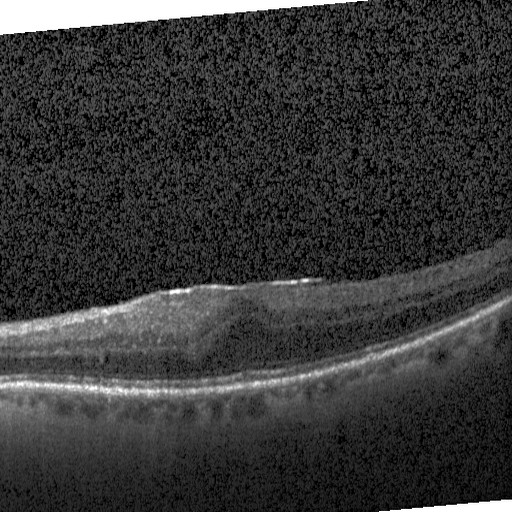
Macular OCT: diabetic macular edema (DME).